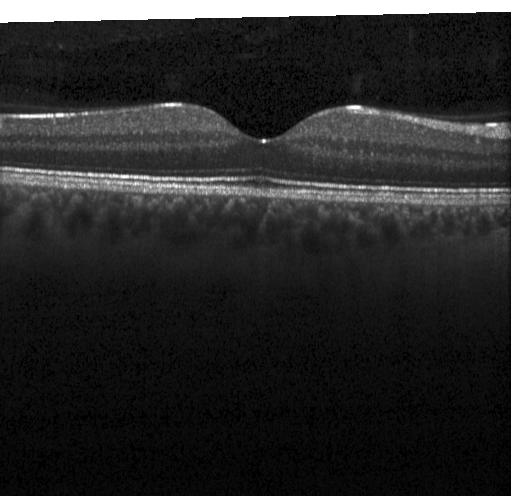
Spectral-domain optical coherence tomography, optical coherence tomography B-scan, Heidelberg Spectralis OCT system, through the macula. Finding: no choroidal neovascularization, diabetic macular edema, or drusen.